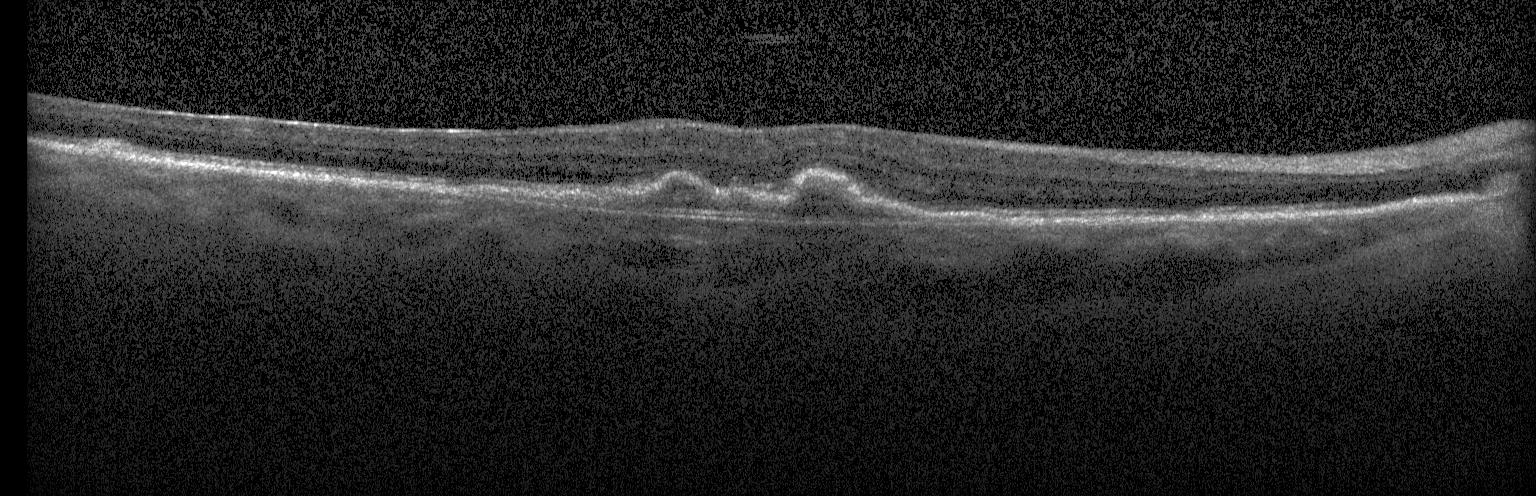
Instrument: Heidelberg Spectralis; through the macula; optical coherence tomography scan; spectral-domain optical coherence tomography.
OCT finding: a choroidal neovascular membrane.